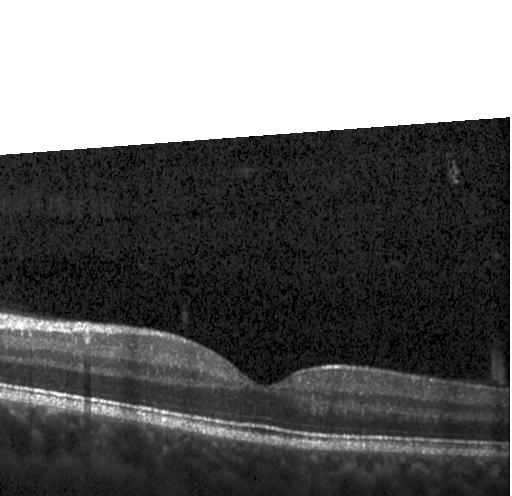
OCT scan showing neither CNV, DME, nor drusen.